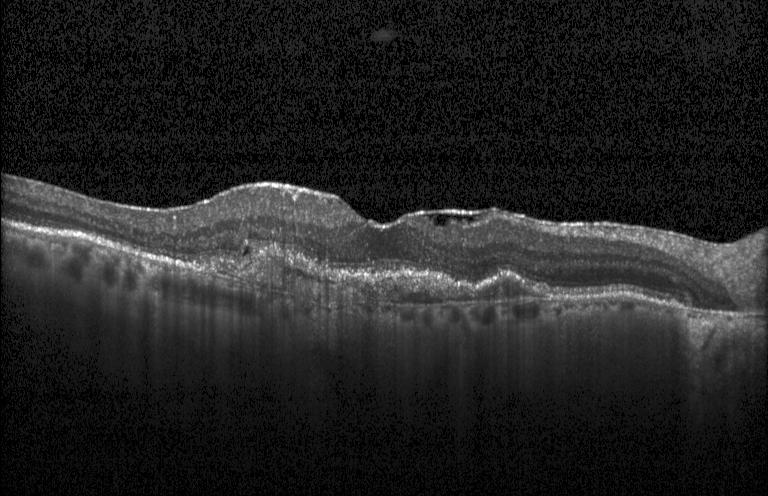 Optical coherence tomography scan. Through the macula. Spectral-domain optical coherence tomography. Heidelberg Spectralis — OCT finding: a choroidal neovascular membrane.